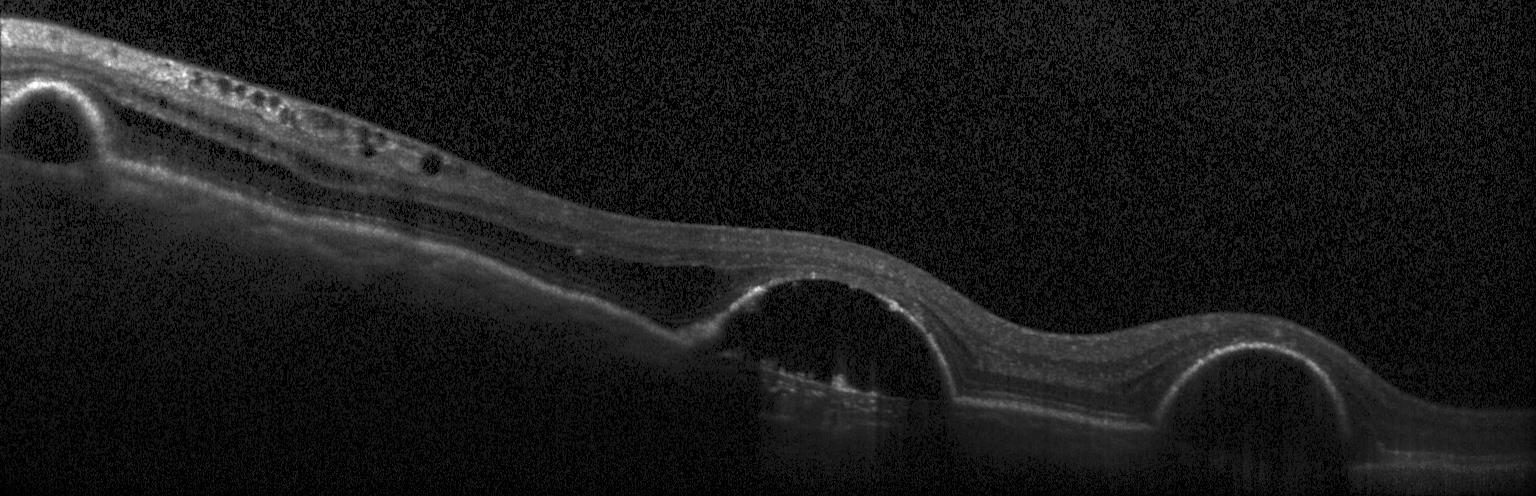 OCT line scan.
OCT finding: a choroidal neovascular membrane.